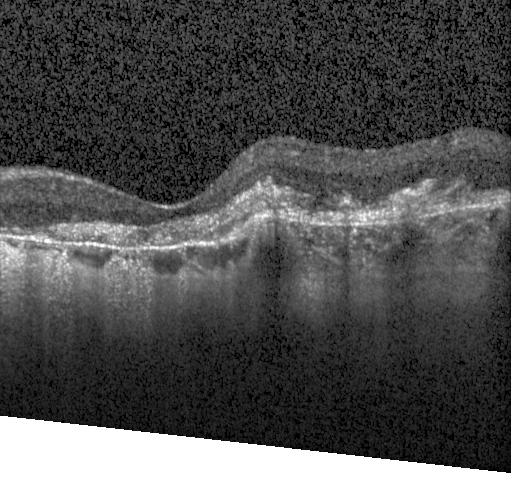

Retinal OCT cross-section. Spectral-domain OCT. Macular scan. Finding: choroidal neovascularization.